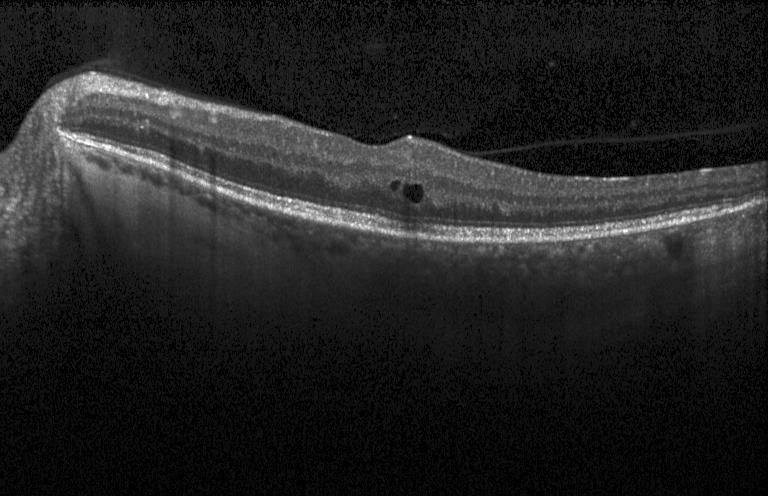 Finding: diabetic macular edema.